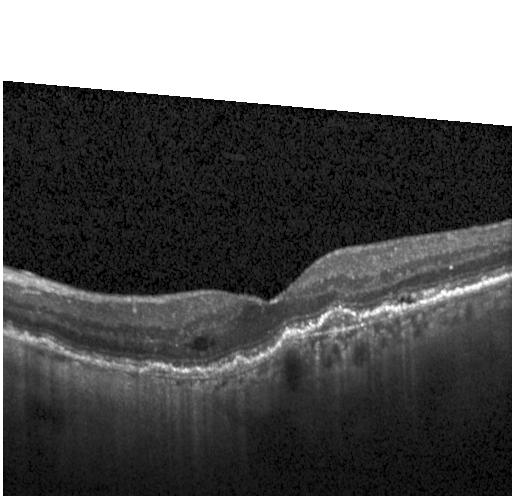
Centered on the fovea. OCT line scan.
The scan shows a choroidal neovascular membrane.